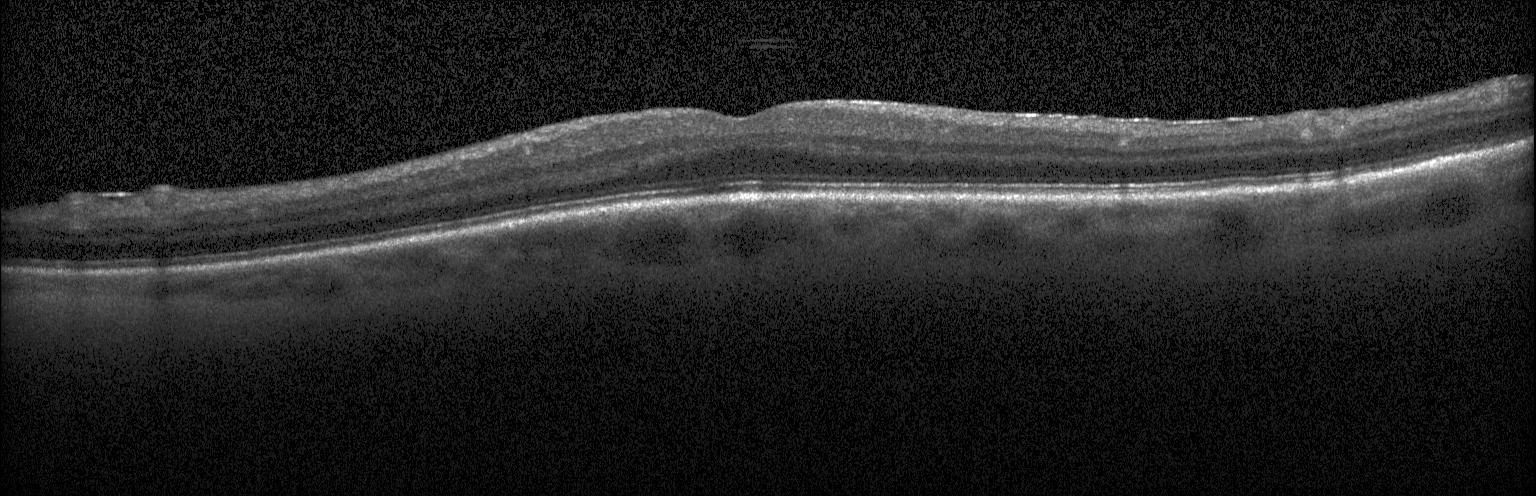 Optical coherence tomography B-scan, horizontal scan through the fovea, Heidelberg Spectralis, spectral-domain optical coherence tomography — No choroidal neovascularization, diabetic macular edema, or drusen.